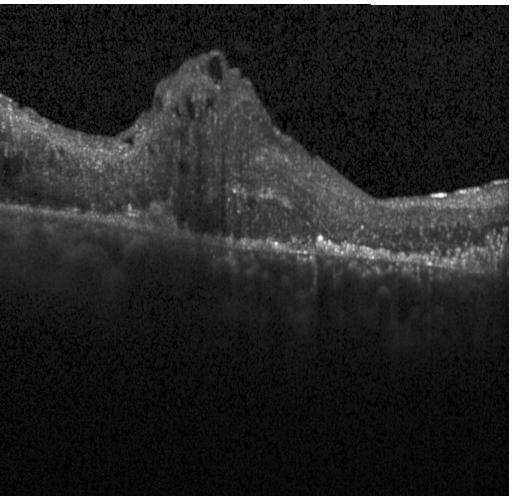 Spectral-domain OCT B-scan: a choroidal neovascular membrane.